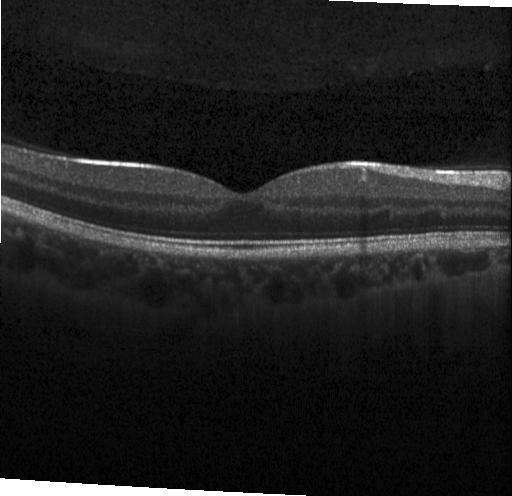

This B-scan demonstrates no CNV, DME, or drusen.